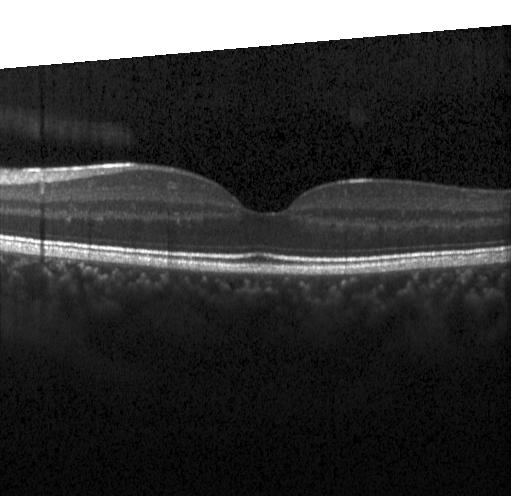

Spectral-domain OCT. Optical coherence tomography B-scan. Instrument: Heidelberg Spectralis
OCT finding: neither CNV, DME, nor drusen.